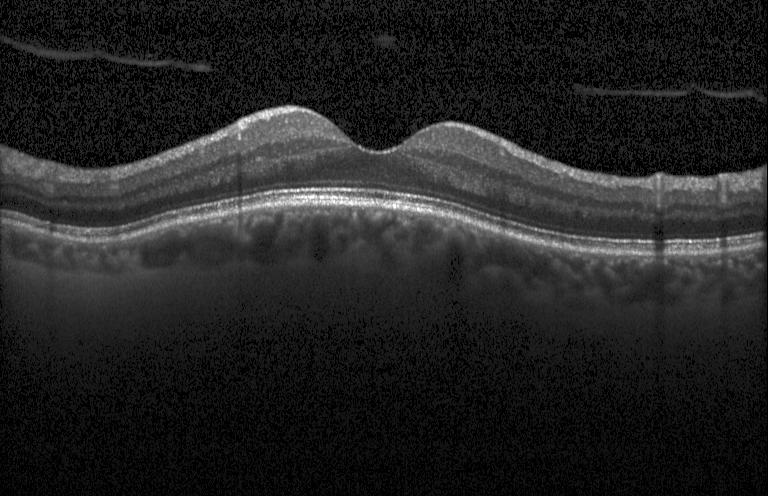
Optical coherence tomography B-scan — No CNV, DME, or drusen.